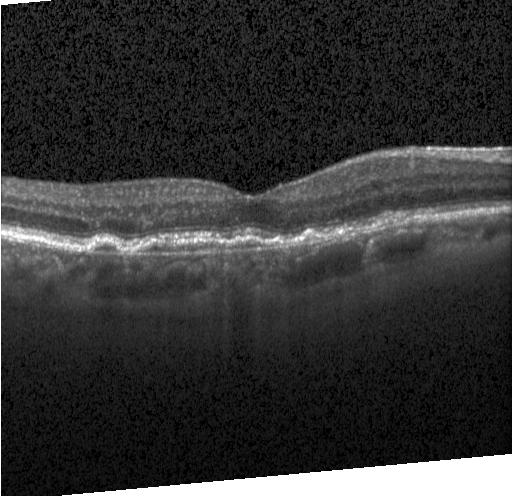
Retinal OCT B-scan.
Macular OCT: a choroidal neovascular membrane.